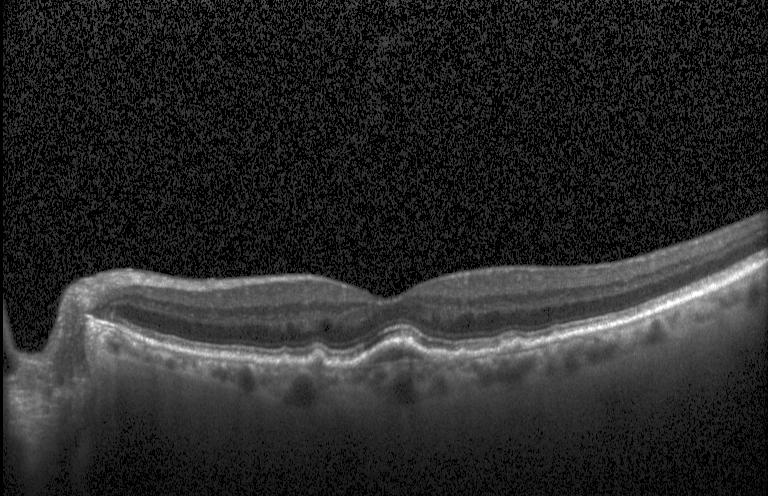 OCT B-scan showing CNV.